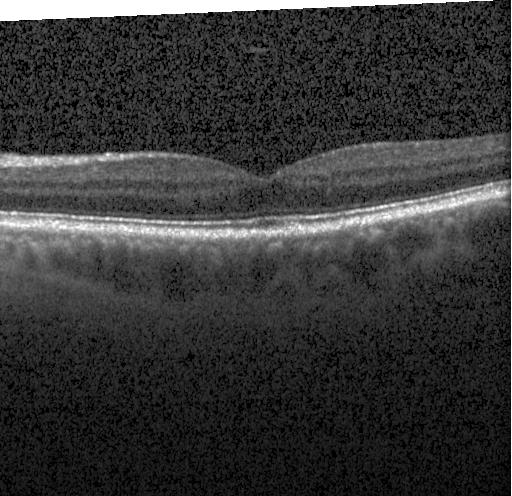
Centered on the fovea, acquired on a Heidelberg Spectralis, optical coherence tomography B-scan, spectral-domain optical coherence tomography
Finding: no choroidal neovascularization, no diabetic macular edema, and no drusen.